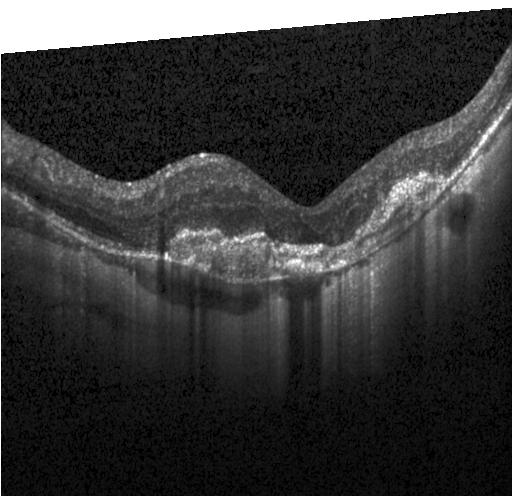 Macular OCT: a choroidal neovascular membrane.